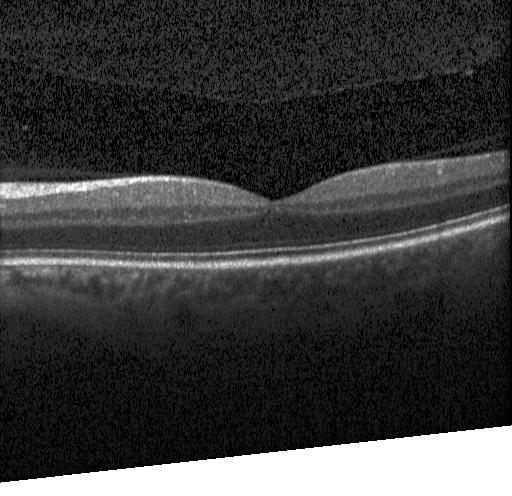
Heidelberg Spectralis. Optical coherence tomography scan. Centered on the fovea.
This B-scan demonstrates no evidence of CNV, DME, or drusen.